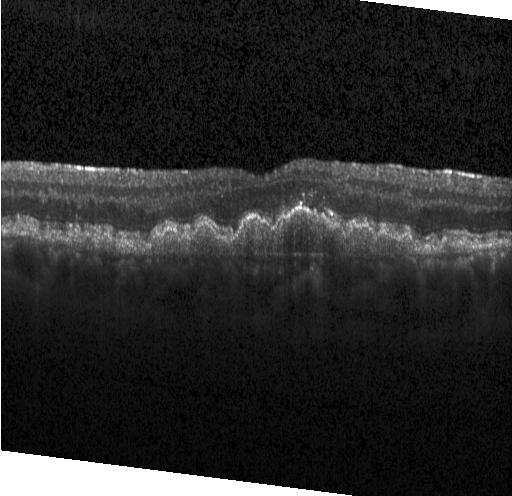 Impression: a choroidal neovascular membrane.